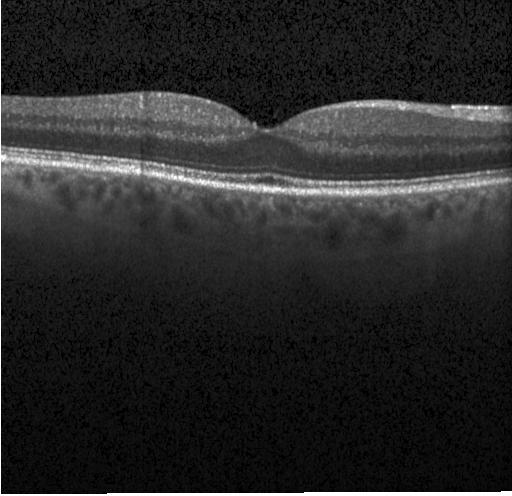

Diagnosis: no choroidal neovascularization, no diabetic macular edema, and no drusen.